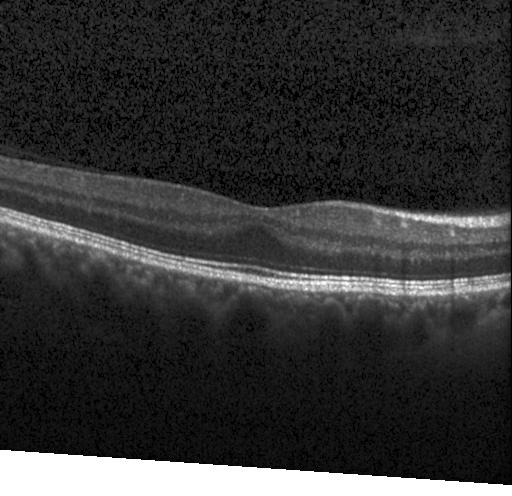

Macular OCT demonstrating neither choroidal neovascularization, diabetic macular edema, nor drusen.